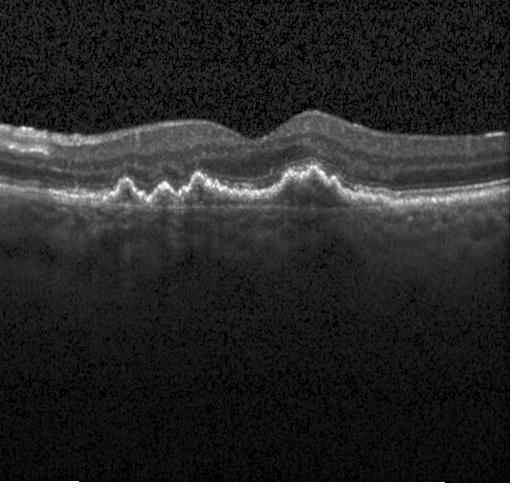
Spectral-domain OCT; OCT line scan
Finding: CNV.